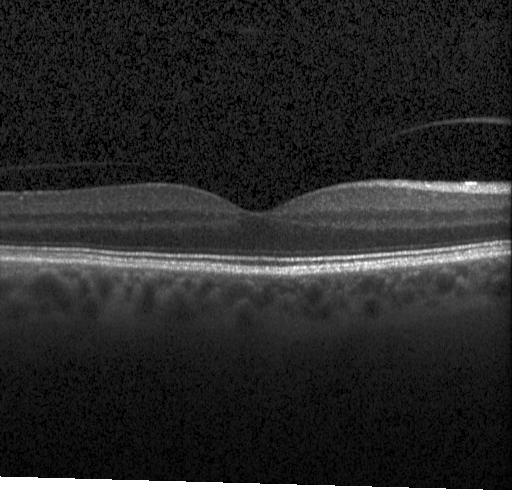

Impression: no evidence of CNV, DME, or drusen.